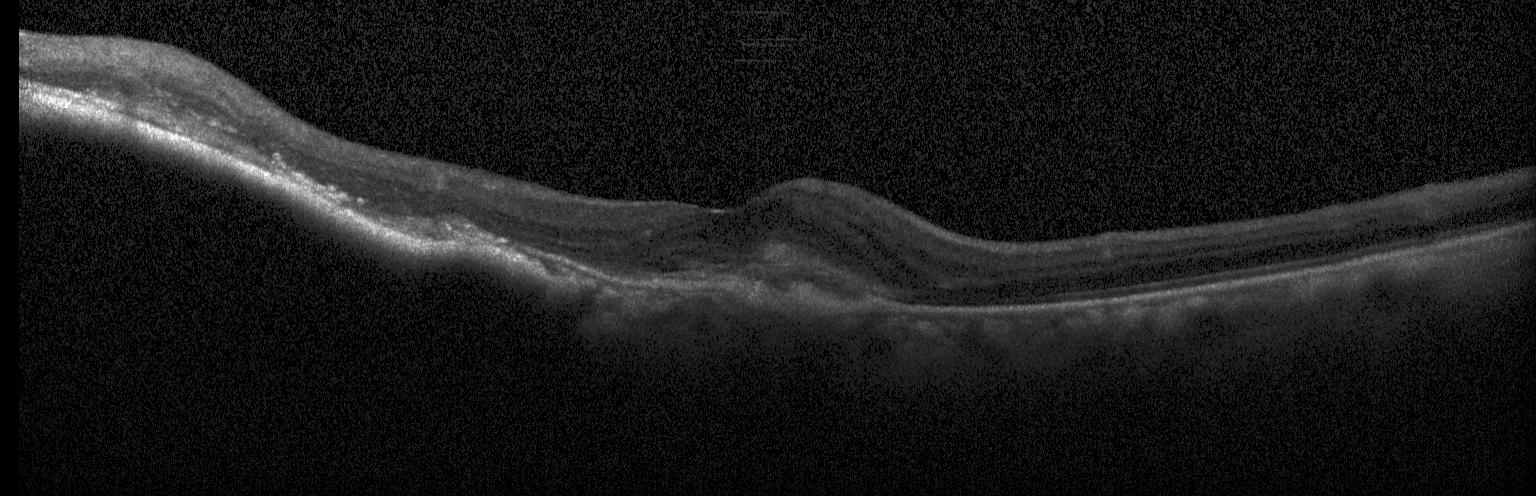
Optical coherence tomography B-scan · instrument: Heidelberg Spectralis.
Impression: a choroidal neovascular membrane.